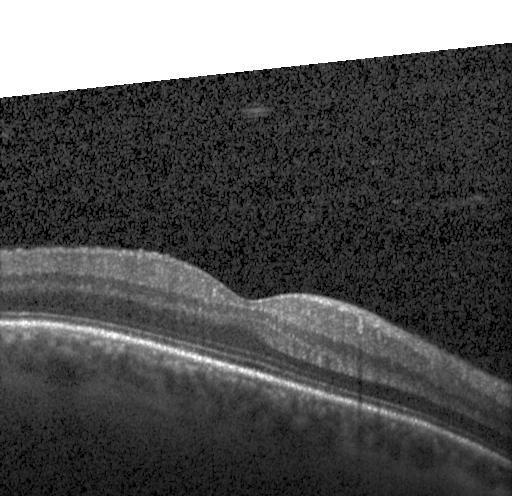 OCT B-scan showing no evidence of CNV, DME, or drusen.